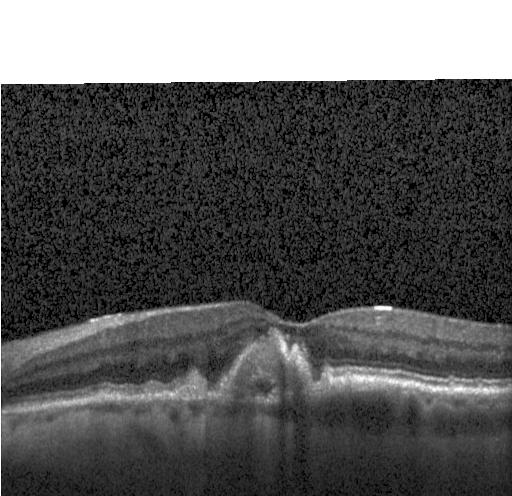

Heidelberg Spectralis, optical coherence tomography B-scan, horizontal scan through the fovea, SD-OCT
Diagnosis: choroidal neovascularization (CNV).